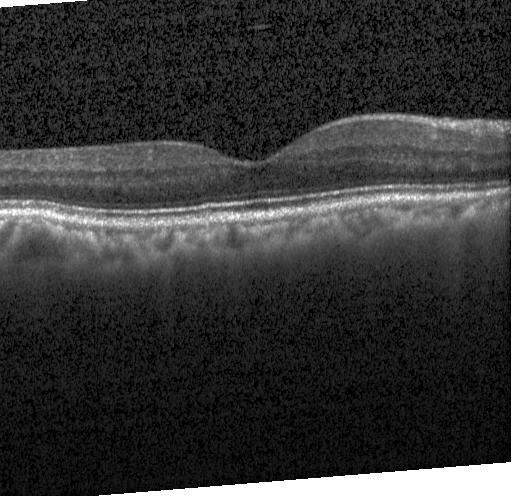 Acquired on a Heidelberg Spectralis, optical coherence tomography scan — No choroidal neovascularization, no diabetic macular edema, and no drusen.